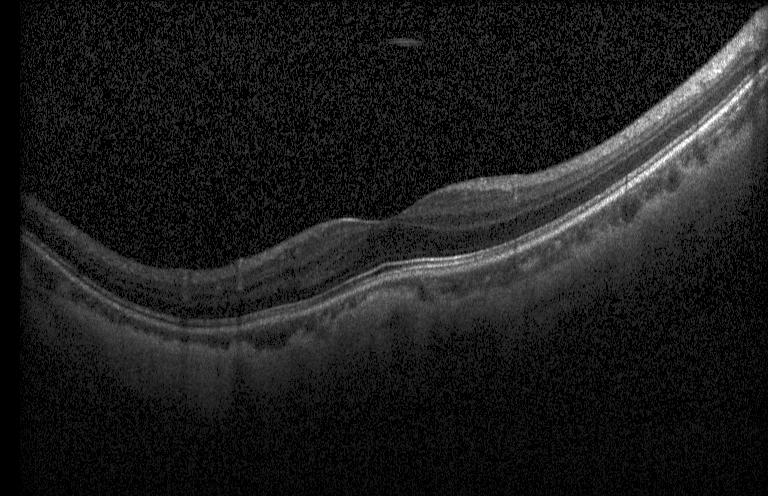

OCT finding: no choroidal neovascularization, no diabetic macular edema, and no drusen.